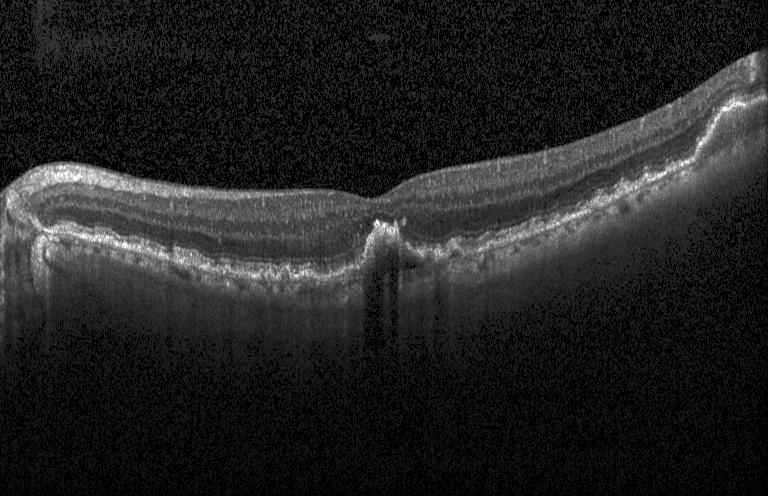 Assessment: a choroidal neovascular membrane.